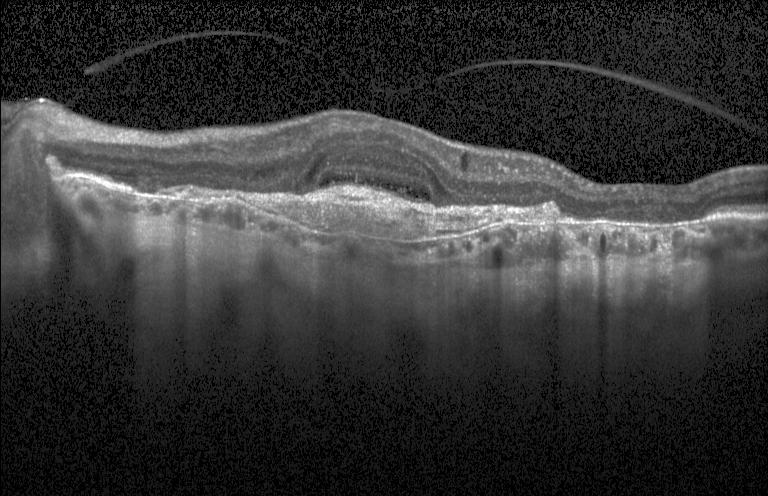

OCT scan showing choroidal neovascularization (CNV).